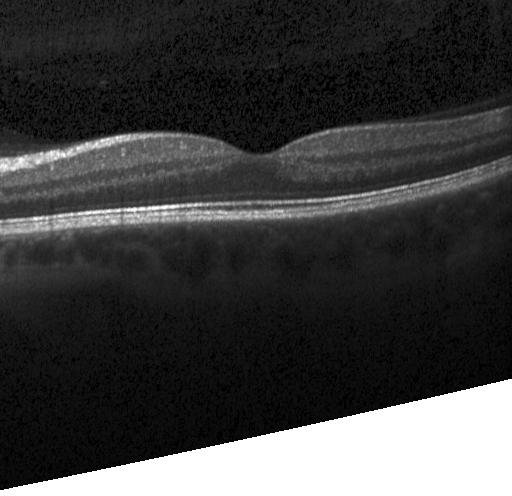

Fovea-centered, instrument: Heidelberg Spectralis, OCT B-scan — Impression: neither choroidal neovascularization, diabetic macular edema, nor drusen.